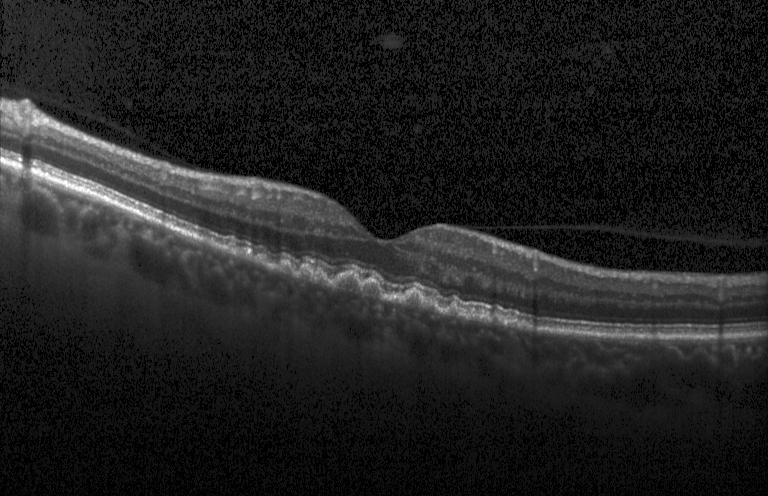

OCT line scan. Finding: drusen.